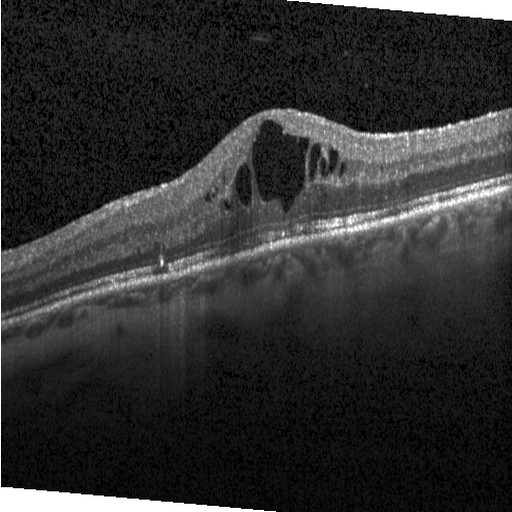
OCT line scan · Heidelberg Spectralis · SD-OCT · macular scan.
Diagnosis: diabetic macular edema.